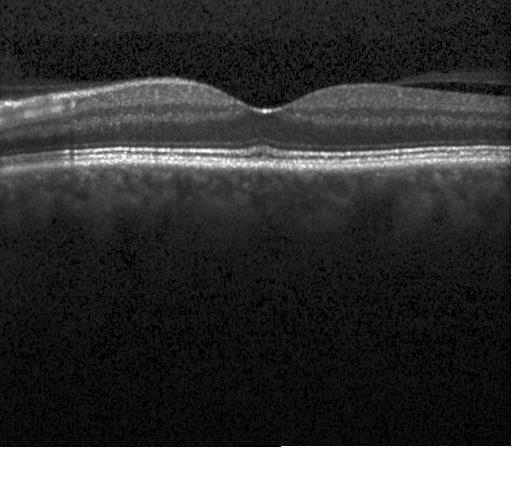 Retinal OCT B-scan; instrument: Heidelberg Spectralis
Impression: neither CNV, DME, nor drusen.